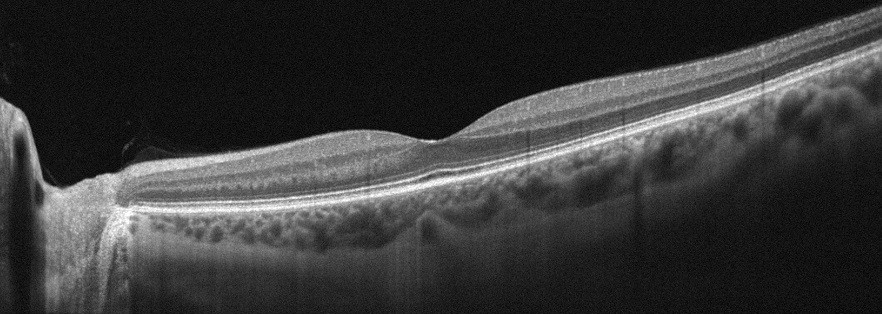
Retinal OCT B-scan. Instrument: Optovue Avanti RTVue XR — This B-scan demonstrates no AMD, DME, ERM, RAO, RVO, or VID.